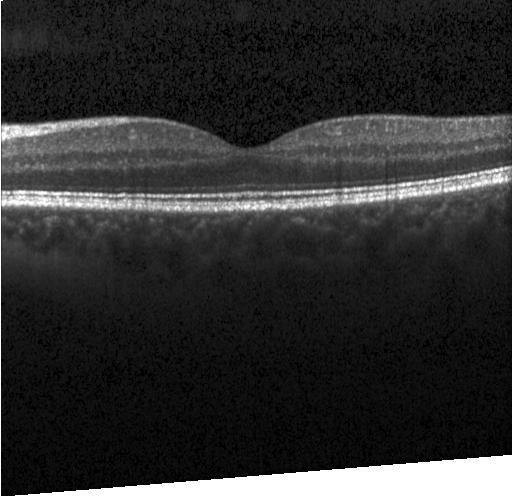 OCT B-scan showing no choroidal neovascularization, diabetic macular edema, or drusen.